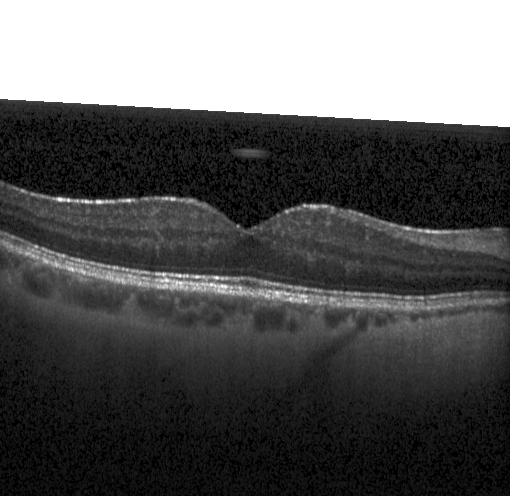 The scan shows no evidence of choroidal neovascularization, diabetic macular edema, or drusen.